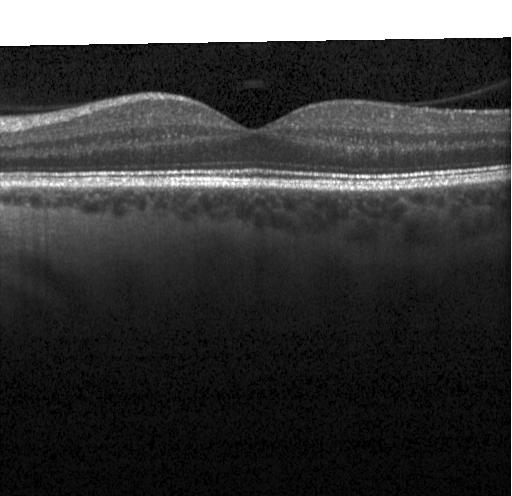
Instrument: Heidelberg Spectralis, retinal OCT cross-section, horizontal scan through the fovea, spectral-domain optical coherence tomography.
Finding: no choroidal neovascularization, diabetic macular edema, or drusen.